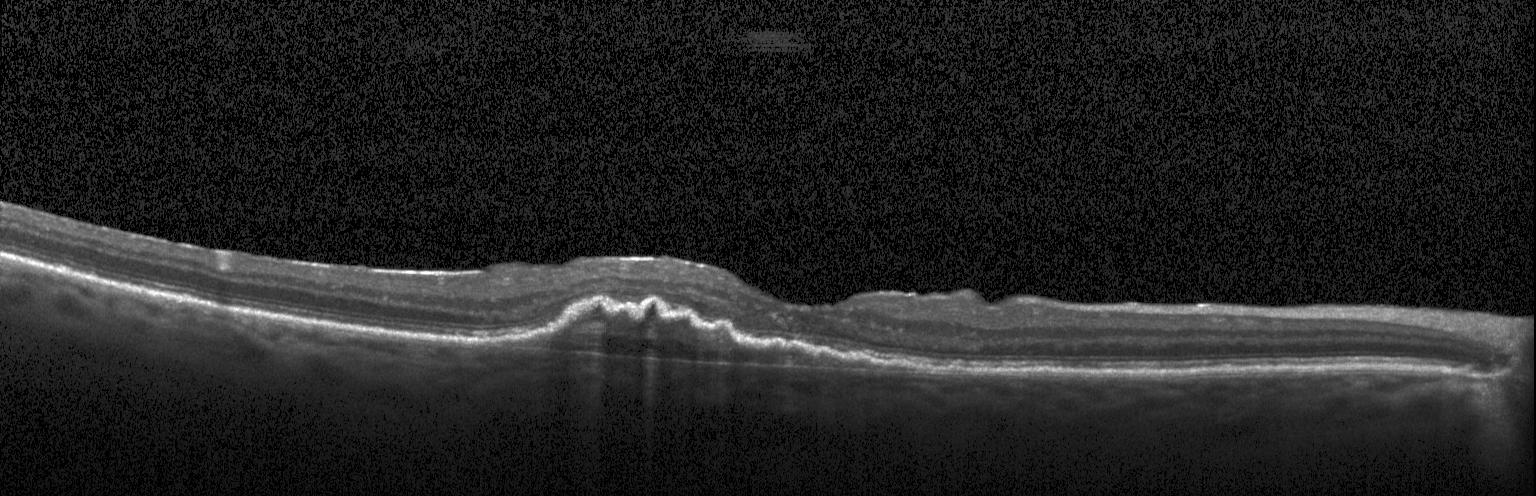

Optical coherence tomography scan. Finding: choroidal neovascularization (CNV).